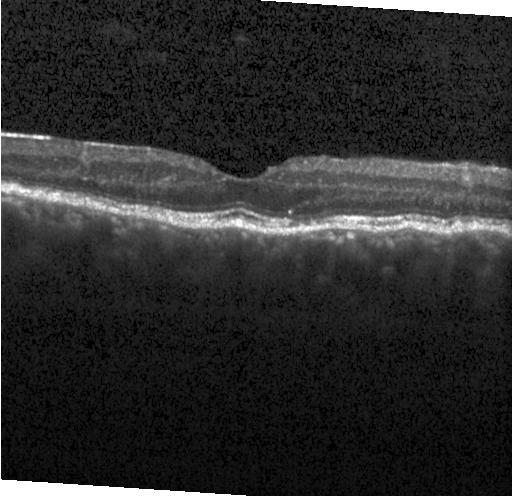 OCT finding: no evidence of choroidal neovascularization, diabetic macular edema, or drusen.